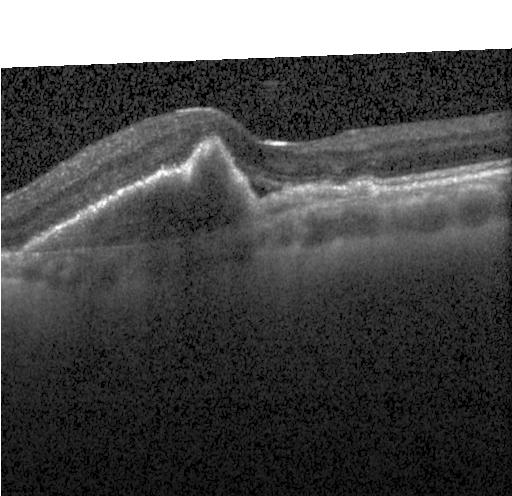
This B-scan demonstrates choroidal neovascularization.